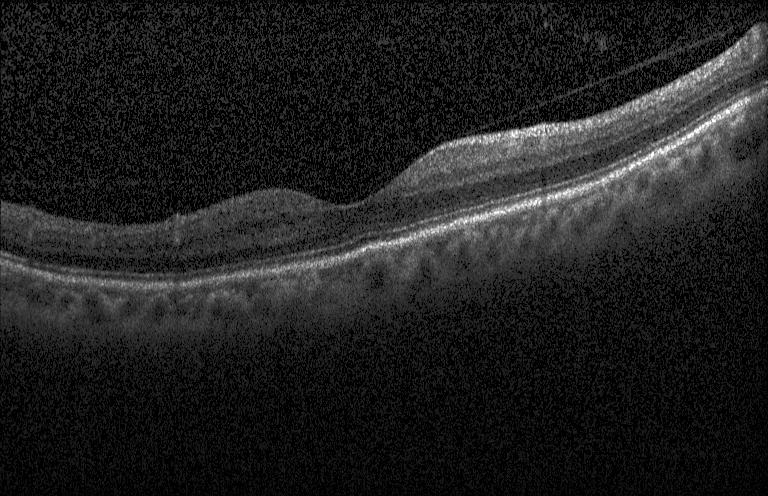

Retinal OCT B-scan. Acquired on a Heidelberg Spectralis. Horizontal scan through the fovea. Spectral-domain OCT.
Impression: no choroidal neovascularization, no diabetic macular edema, and no drusen.